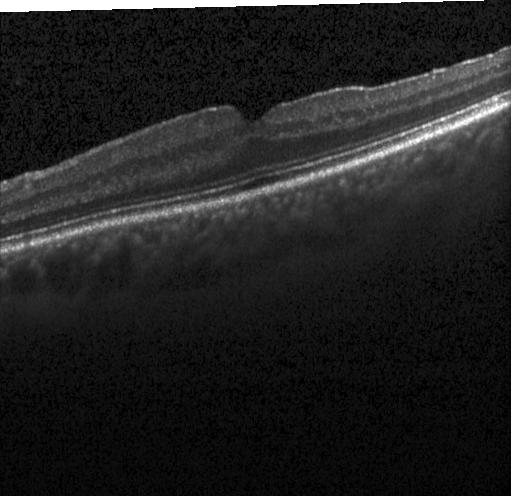 Spectral-domain OCT; horizontal scan through the fovea; retinal OCT cross-section — Assessment: no choroidal neovascularization, diabetic macular edema, or drusen.